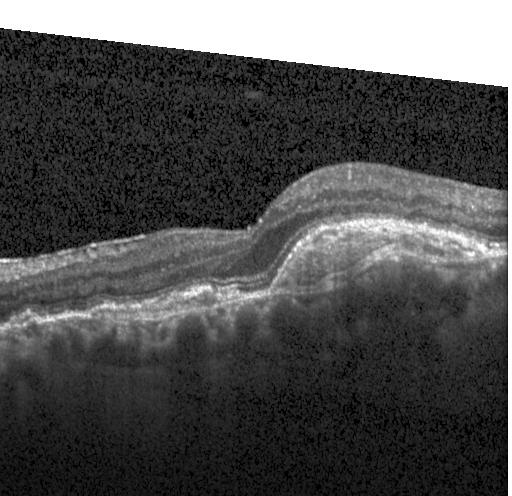

SD-OCT; retinal OCT B-scan; macular scan — This B-scan demonstrates choroidal neovascularization.